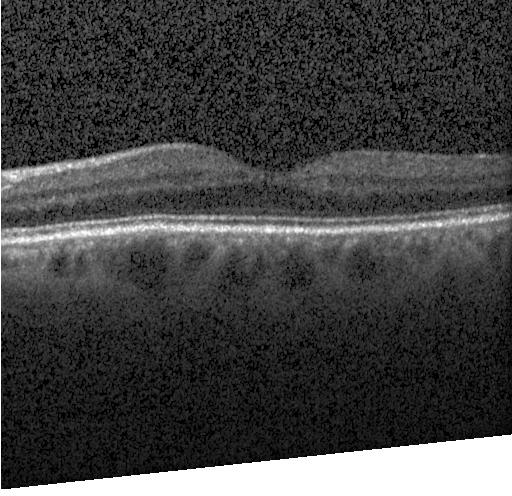

Centered on the fovea · instrument: Heidelberg Spectralis · retinal OCT cross-section — Diagnosis: no CNV, no DME, and no drusen.